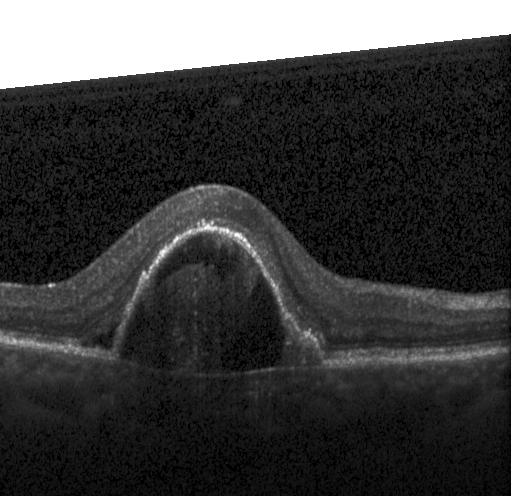 Optical coherence tomography B-scan.
Dx: a choroidal neovascular membrane.